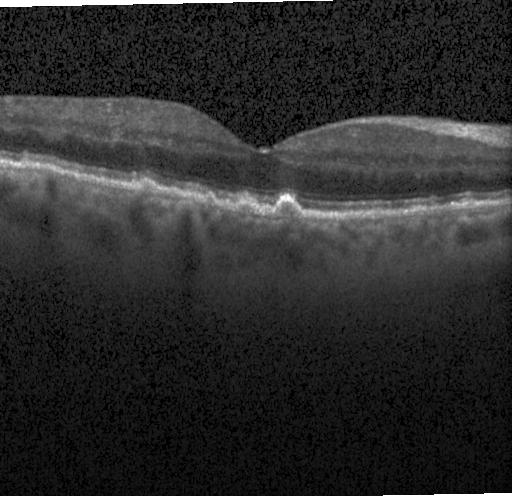

Instrument: Heidelberg Spectralis; OCT B-scan; spectral-domain OCT.
Diagnosis: multiple drusen.